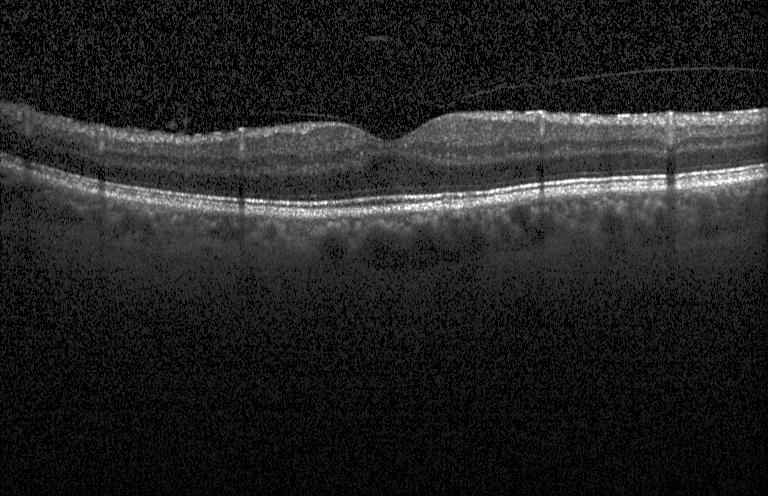
Retinal OCT B-scan. Diagnosis: no CNV, DME, or drusen.